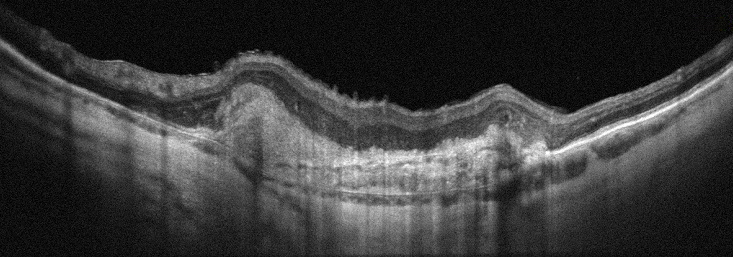

Optical coherence tomography B-scan — Diagnosis: AMD.